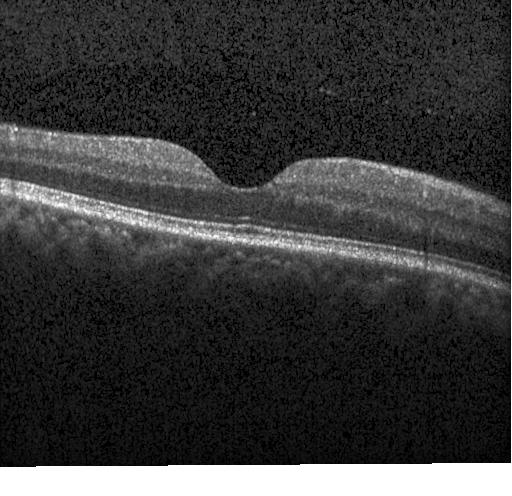

OCT scan showing no choroidal neovascularization, no diabetic macular edema, and no drusen.